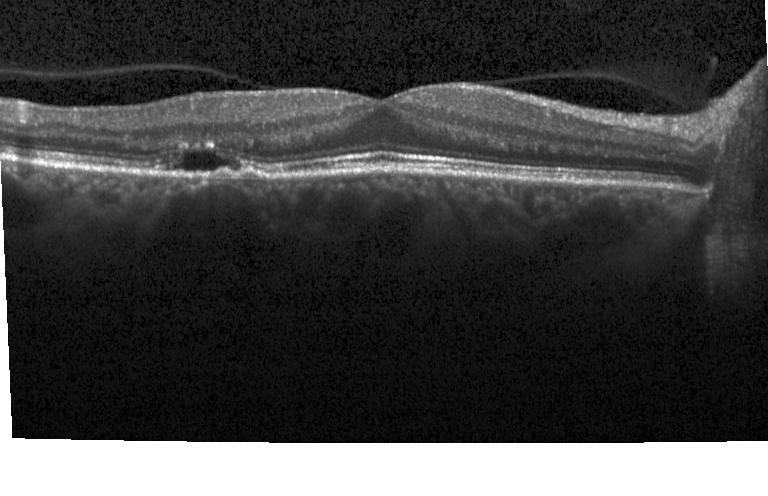

Optical coherence tomography B-scan — Diagnosis: a choroidal neovascular membrane.